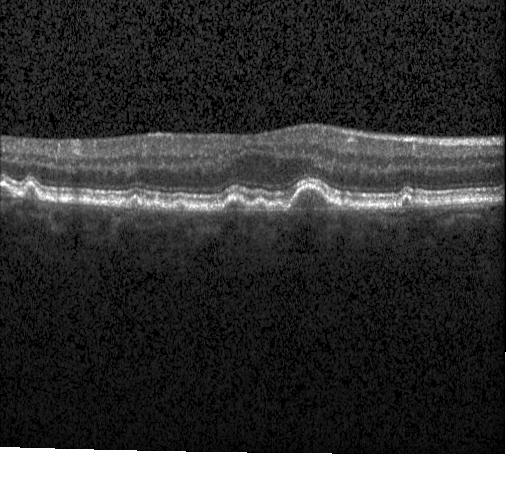 Heidelberg Spectralis; retinal OCT B-scan
Impression: sub-RPE drusenoid deposits.